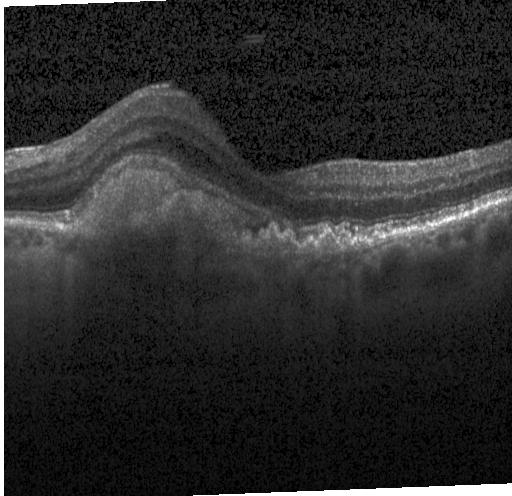
The scan shows choroidal neovascularization.